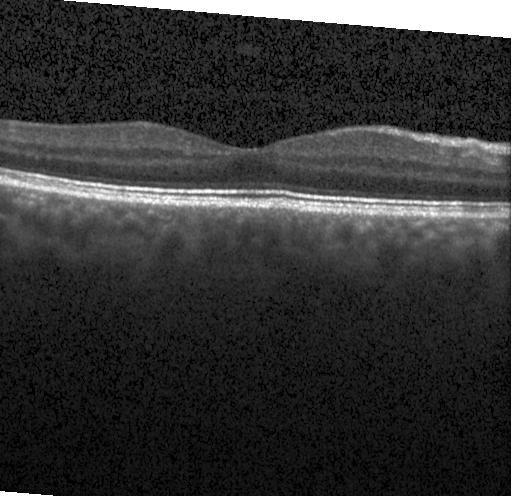

Finding: neither choroidal neovascularization, diabetic macular edema, nor drusen.